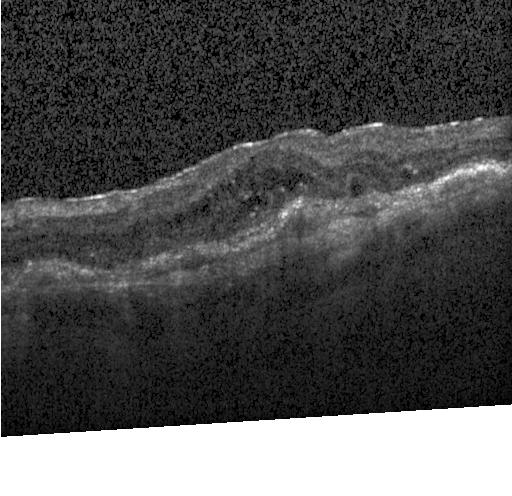

Retinal OCT cross-section · through the macula — Macular OCT: CNV.